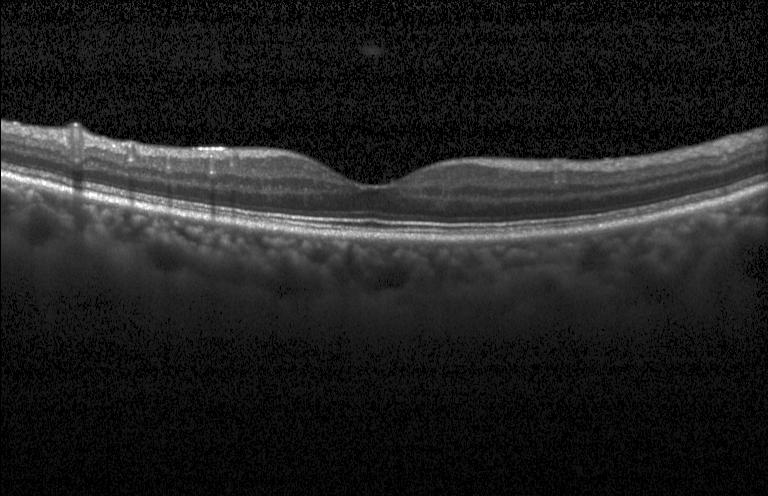 OCT scan showing no evidence of choroidal neovascularization, diabetic macular edema, or drusen.